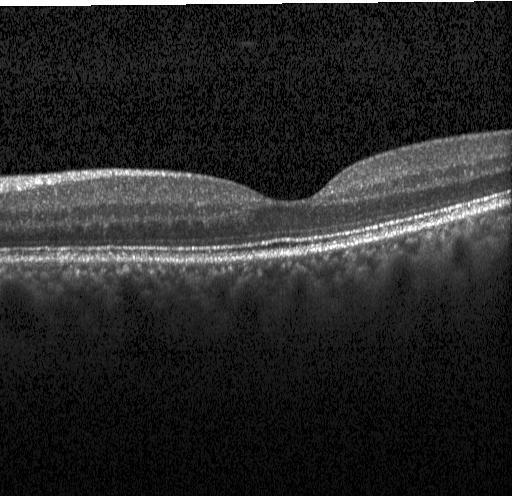
Retinal OCT cross-section; Heidelberg Spectralis OCT system — Diagnosis: neither CNV, DME, nor drusen.